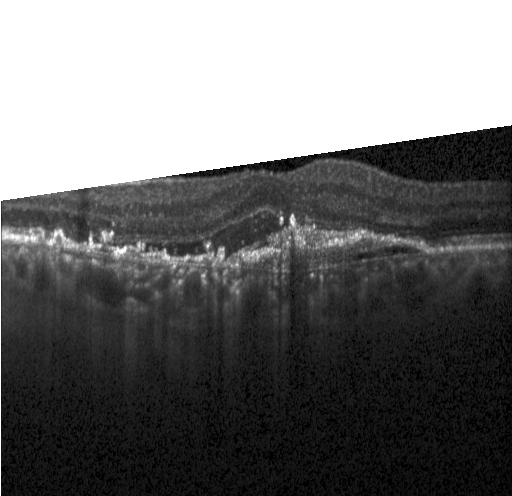
Retinal OCT B-scan, through the macula, spectral-domain optical coherence tomography.
The scan shows a choroidal neovascular membrane.